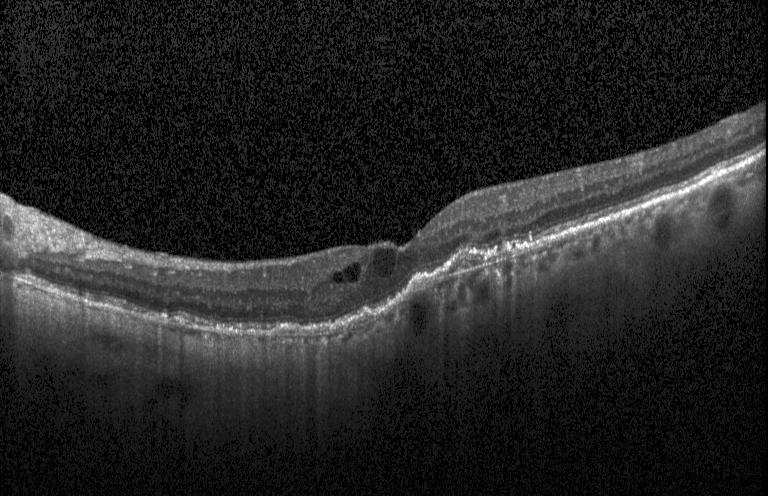
Spectral-domain OCT. Through the macula. Retinal OCT cross-section
A choroidal neovascular membrane.